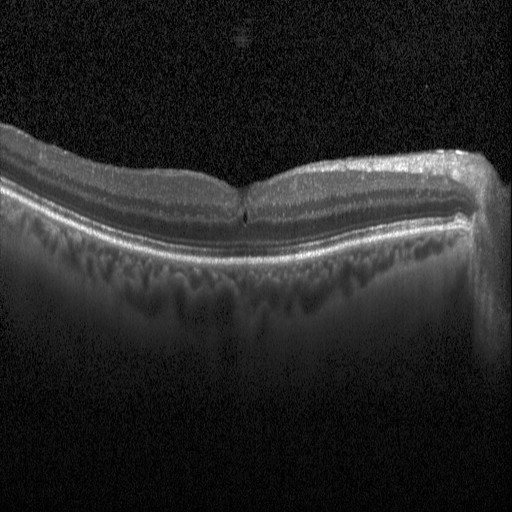 Centered on the fovea, instrument: Heidelberg Spectralis, spectral-domain OCT, retinal OCT cross-section. Assessment: diabetic macular edema.